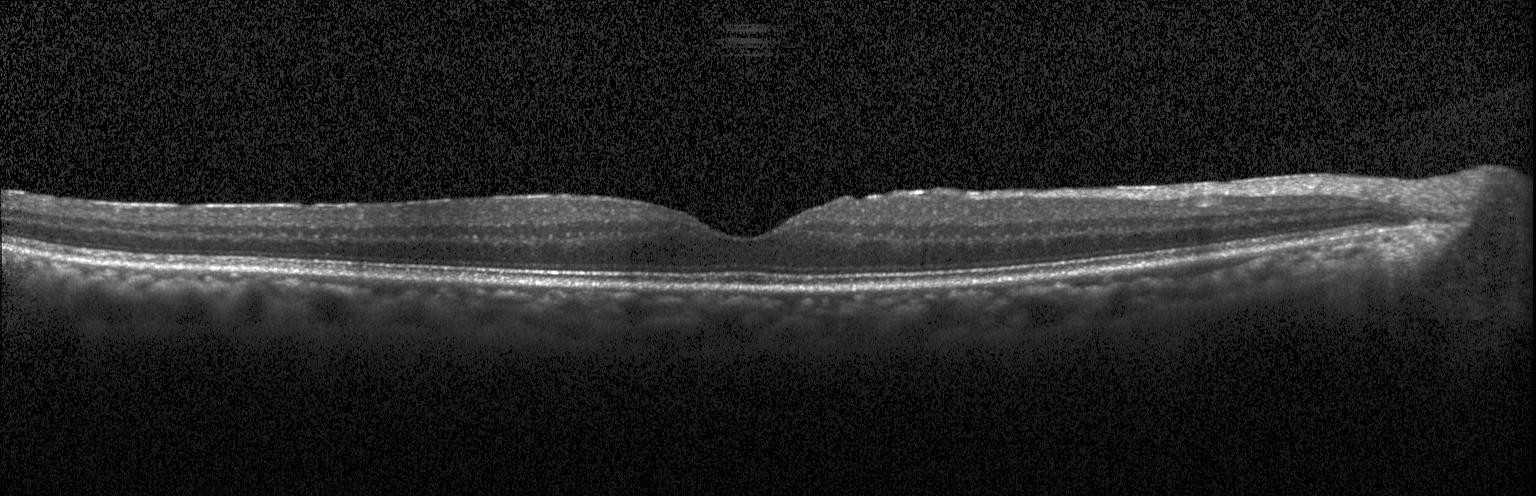

Heidelberg Spectralis, SD-OCT, retinal OCT cross-section, macular scan — Diagnosis: no evidence of choroidal neovascularization, diabetic macular edema, or drusen.